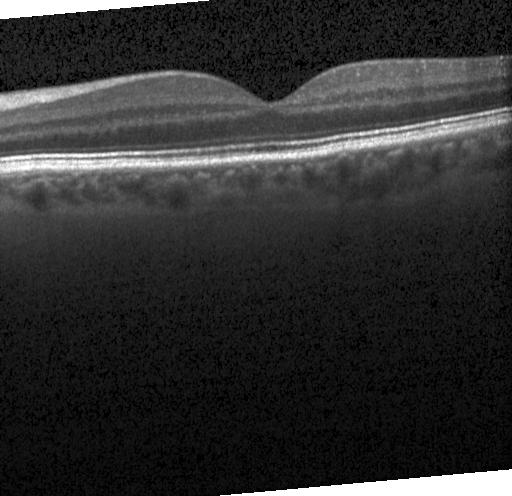 Finding: no CNV, no DME, and no drusen.